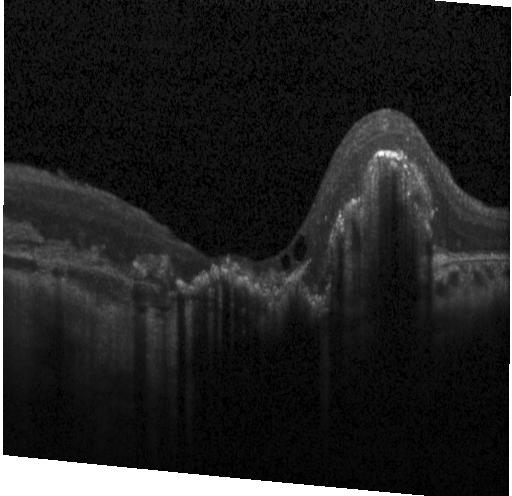 Impression: a choroidal neovascular membrane.